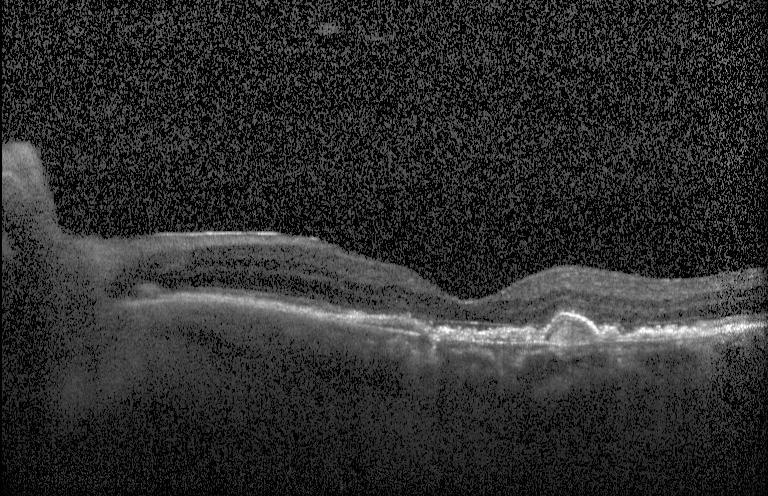 Retinal OCT B-scan
Impression: a choroidal neovascular membrane.